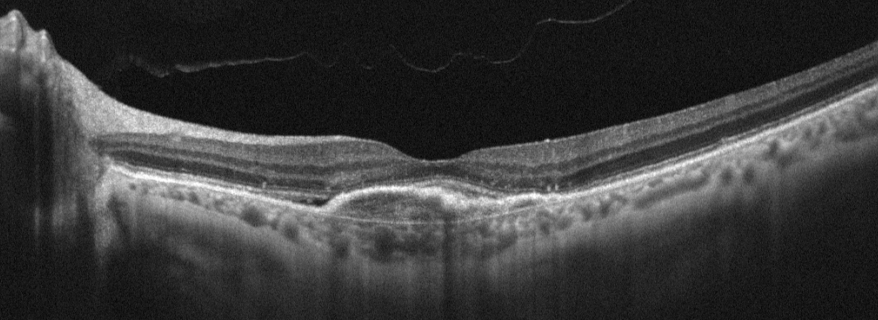 Diagnosis: age-related macular degeneration.